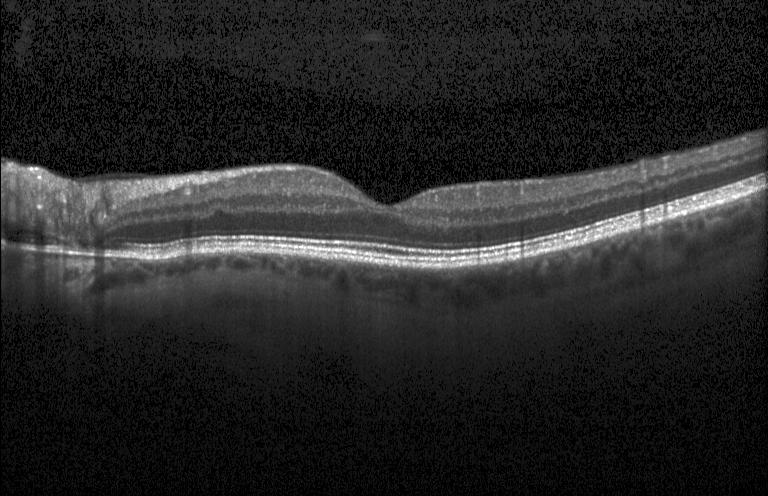

Centered on the fovea, spectral-domain OCT, optical coherence tomography B-scan, Heidelberg Spectralis OCT system
Dx: neither choroidal neovascularization, diabetic macular edema, nor drusen.